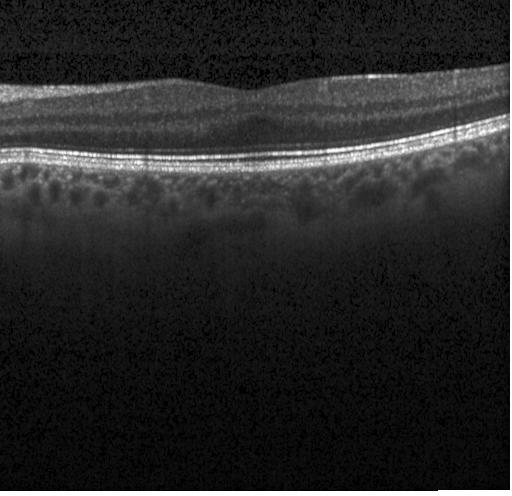

OCT B-scan
Assessment: no choroidal neovascularization, diabetic macular edema, or drusen.